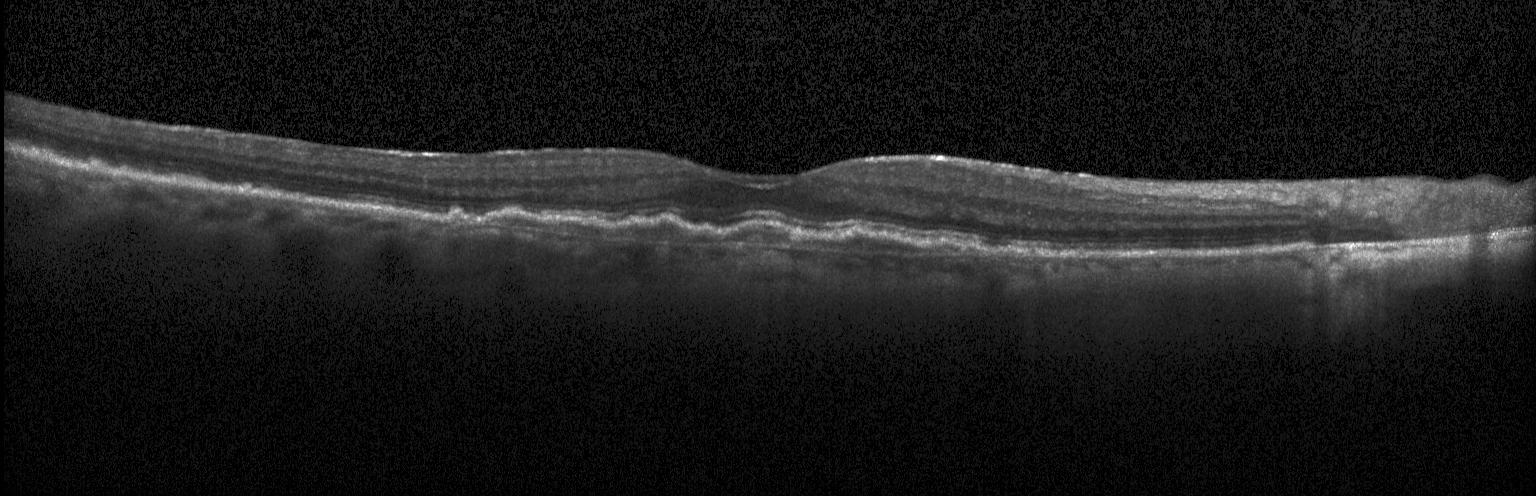 Spectral-domain OCT B-scan: a choroidal neovascular membrane.